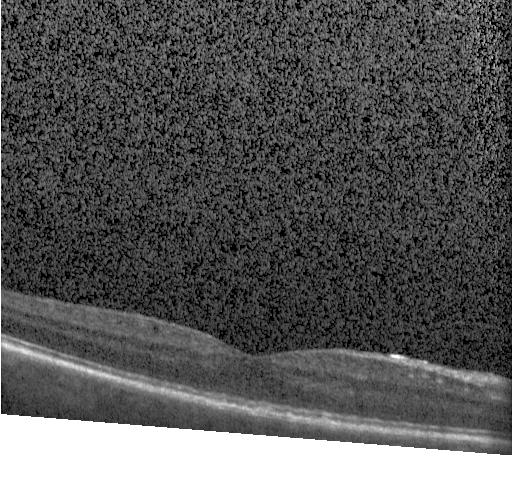

Spectral-domain OCT, optical coherence tomography B-scan, Heidelberg Spectralis OCT system.
Finding: no choroidal neovascularization, diabetic macular edema, or drusen.